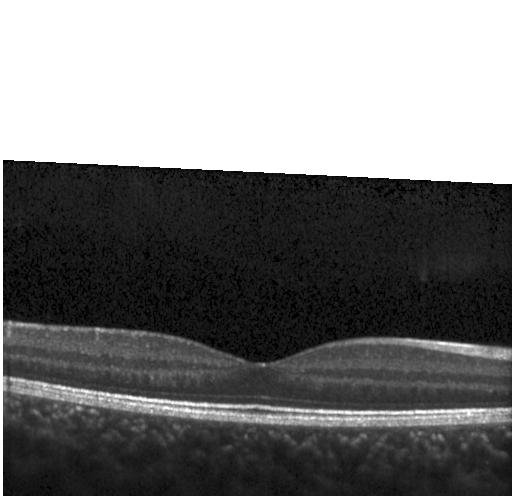 Fovea-centered. Heidelberg Spectralis. Optical coherence tomography B-scan. Assessment: no CNV, no DME, and no drusen.